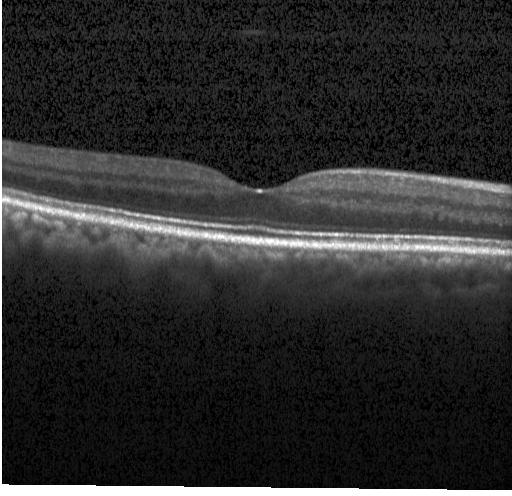

Optical coherence tomography B-scan · spectral-domain optical coherence tomography — Impression: no choroidal neovascularization, no diabetic macular edema, and no drusen.